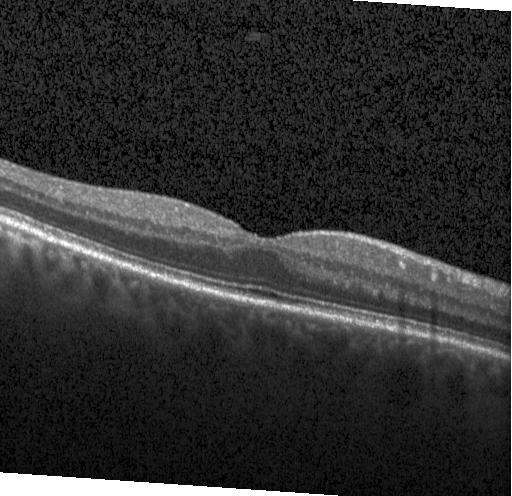
Fovea-centered · instrument: Heidelberg Spectralis · optical coherence tomography scan. Dx: neither choroidal neovascularization, diabetic macular edema, nor drusen.